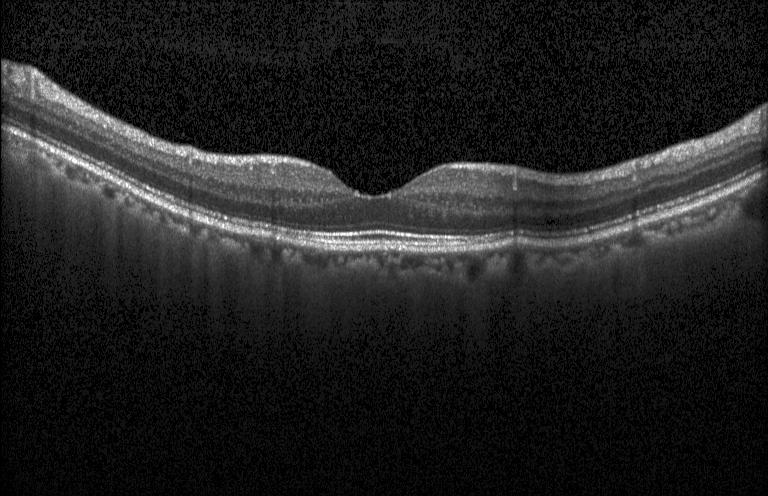

Assessment: no evidence of CNV, DME, or drusen.